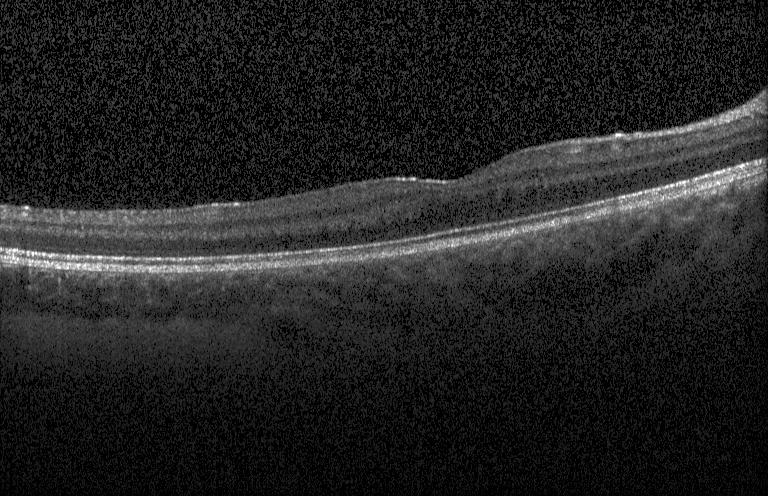
OCT B-scan; spectral-domain optical coherence tomography. Dx: no evidence of CNV, DME, or drusen.